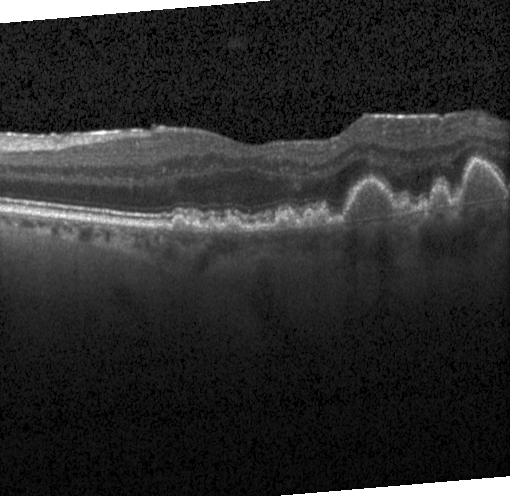

Retinal OCT B-scan; acquired on a Heidelberg Spectralis; spectral-domain OCT; horizontal scan through the fovea
Finding: multiple drusen.